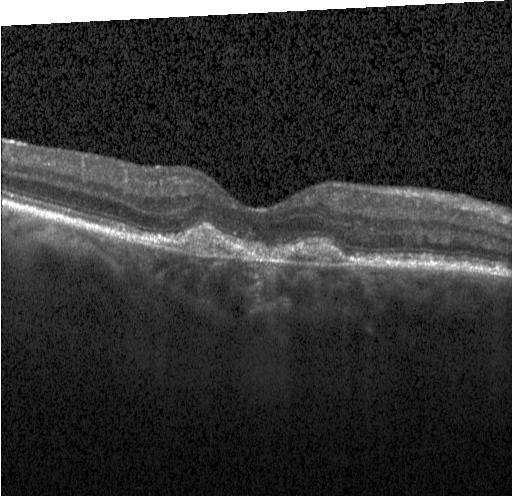

Retinal OCT cross-section
Finding: CNV.